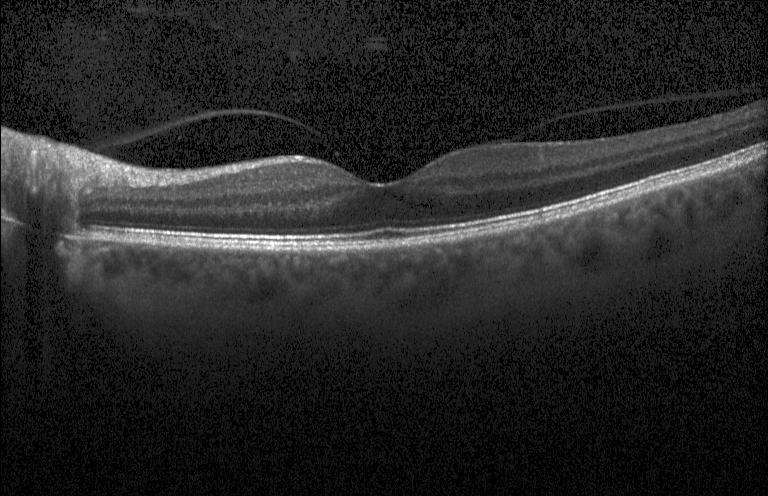

Optical coherence tomography scan, spectral-domain OCT — Dx: no evidence of choroidal neovascularization, diabetic macular edema, or drusen.